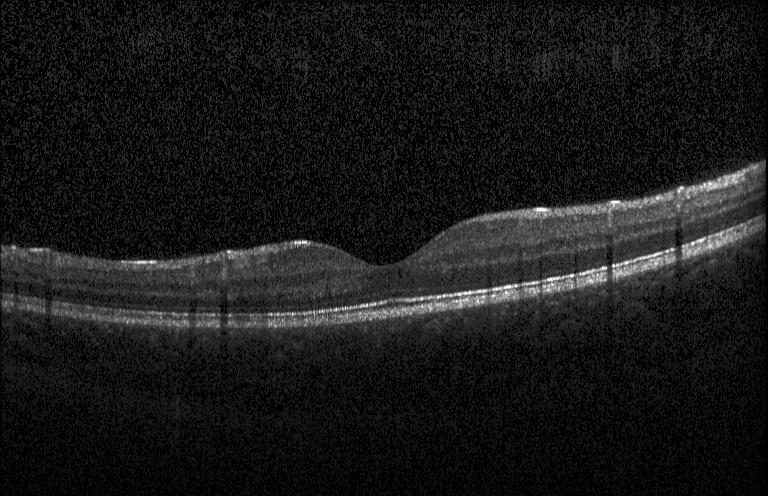

Finding: neither choroidal neovascularization, diabetic macular edema, nor drusen.